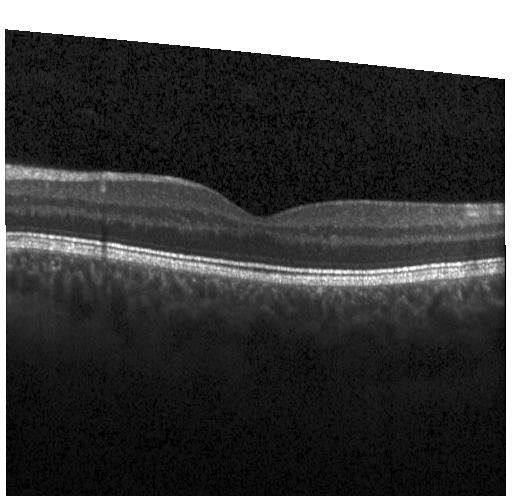 Centered on the fovea, Heidelberg Spectralis, retinal OCT cross-section.
Macular OCT: no CNV, DME, or drusen.